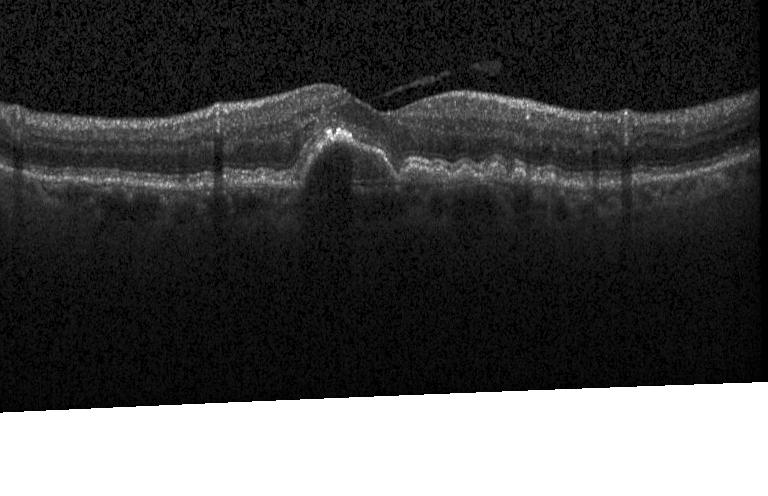

Finding: multiple drusen.